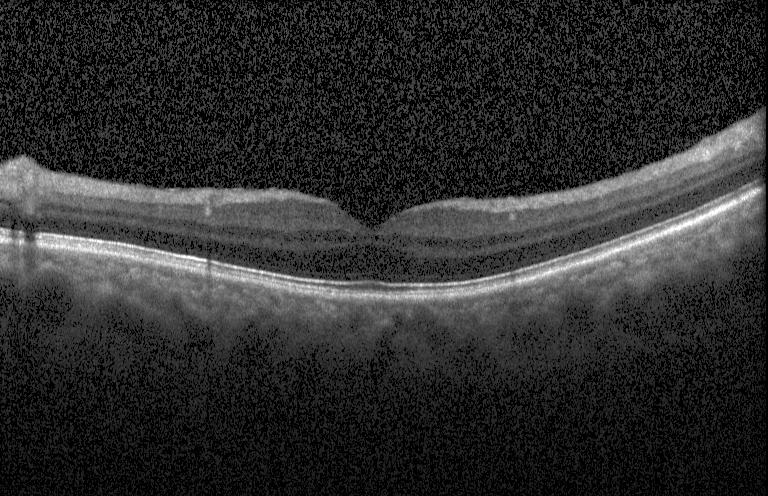

Macular OCT: no evidence of choroidal neovascularization, diabetic macular edema, or drusen.